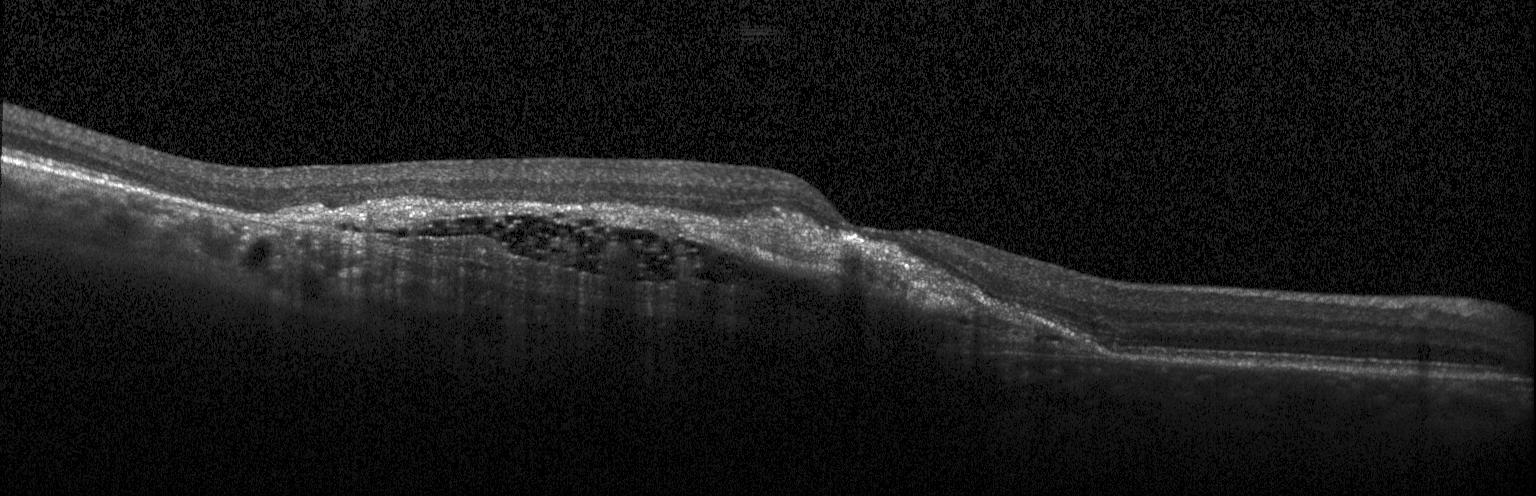
OCT B-scan
Diagnosis: CNV.